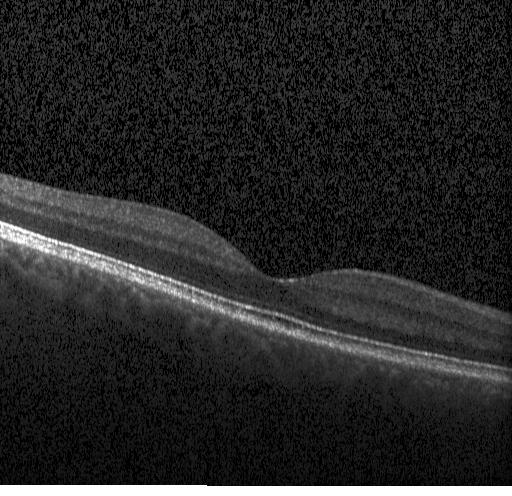

OCT B-scan — Diagnosis: no choroidal neovascularization, diabetic macular edema, or drusen.